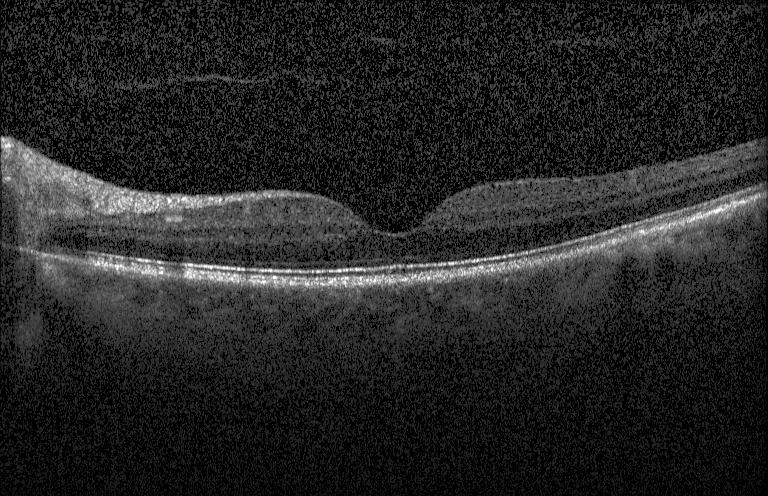
Retinal OCT B-scan. Spectral-domain optical coherence tomography. This B-scan demonstrates no CNV, DME, or drusen.